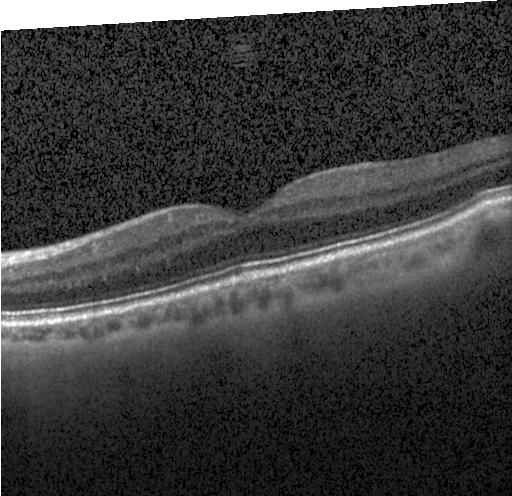
Macular OCT: neither choroidal neovascularization, diabetic macular edema, nor drusen.